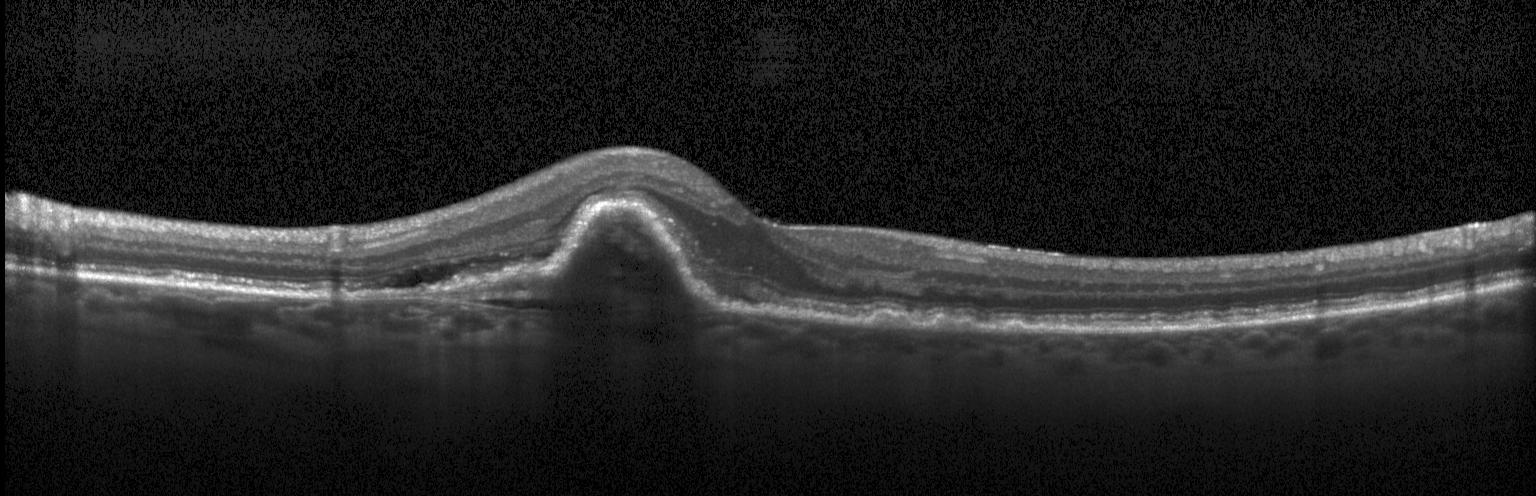 This B-scan demonstrates a choroidal neovascular membrane.